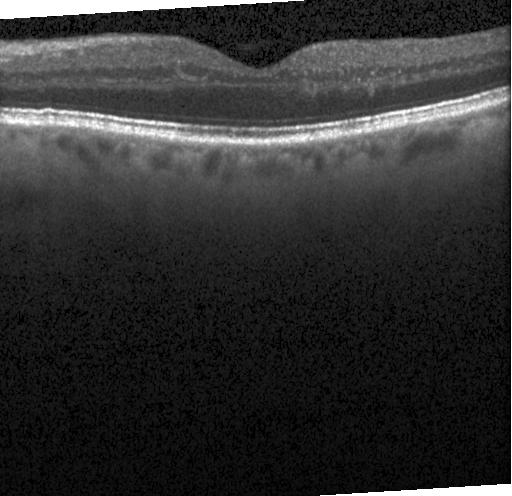
Optical coherence tomography scan. The scan shows no evidence of CNV, DME, or drusen.